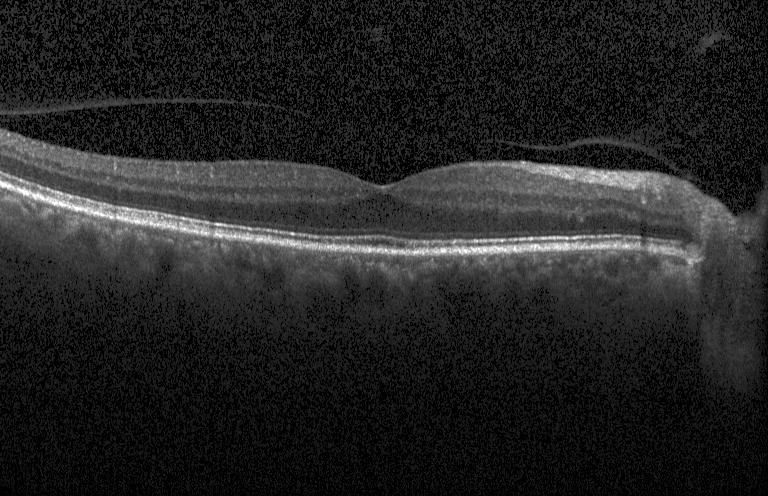 Optical coherence tomography B-scan. Finding: neither CNV, DME, nor drusen.